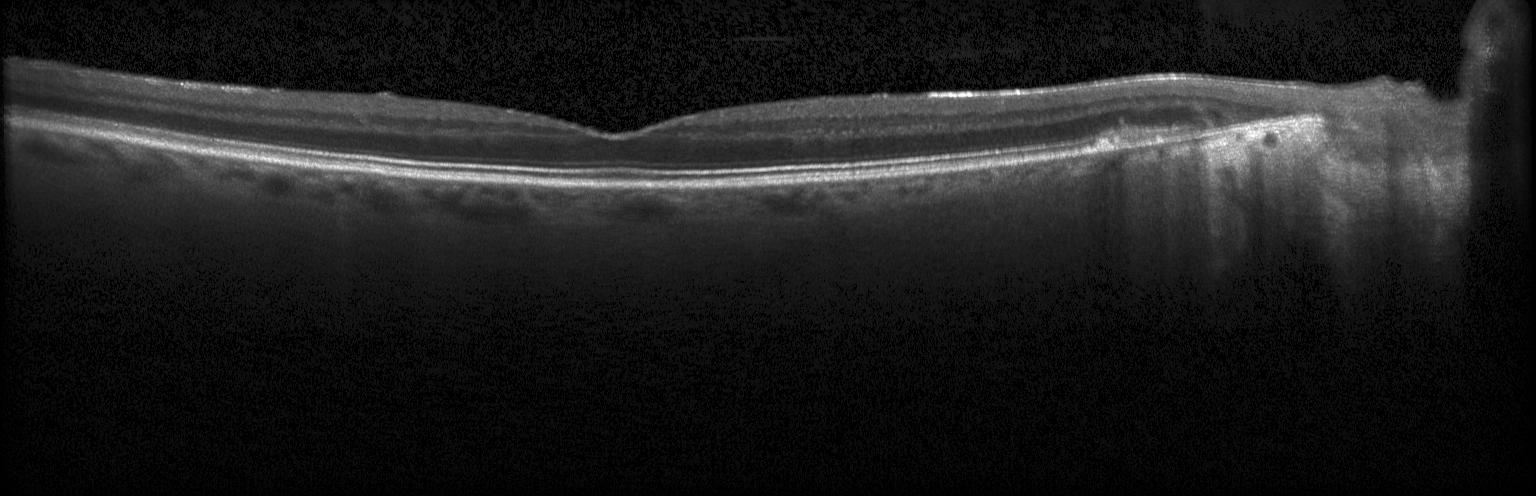 Diagnosis: no CNV, DME, or drusen.